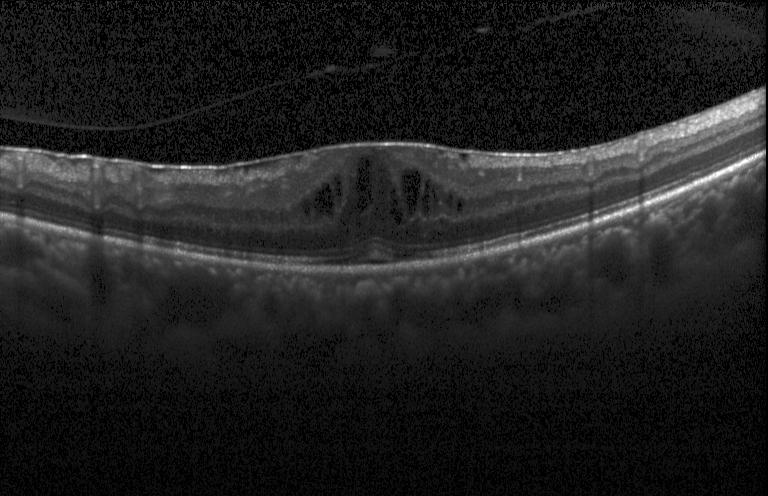
Retinal OCT B-scan · SD-OCT.
Impression: DME.